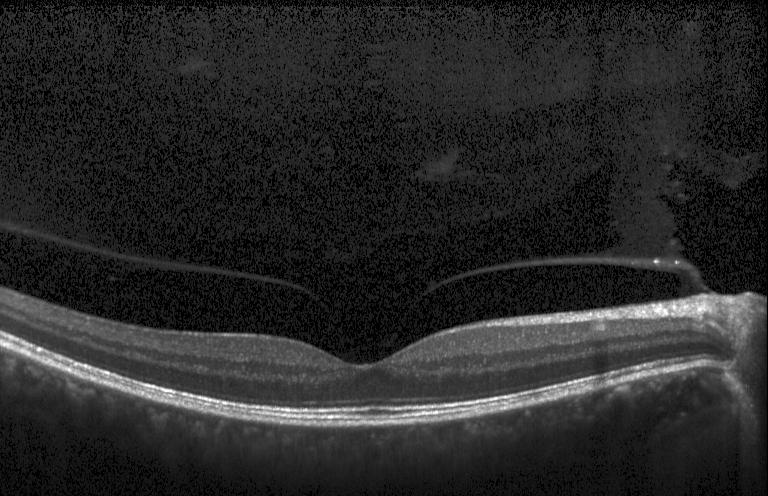

Centered on the fovea, retinal OCT cross-section, Heidelberg Spectralis, SD-OCT
OCT finding: no CNV, DME, or drusen.